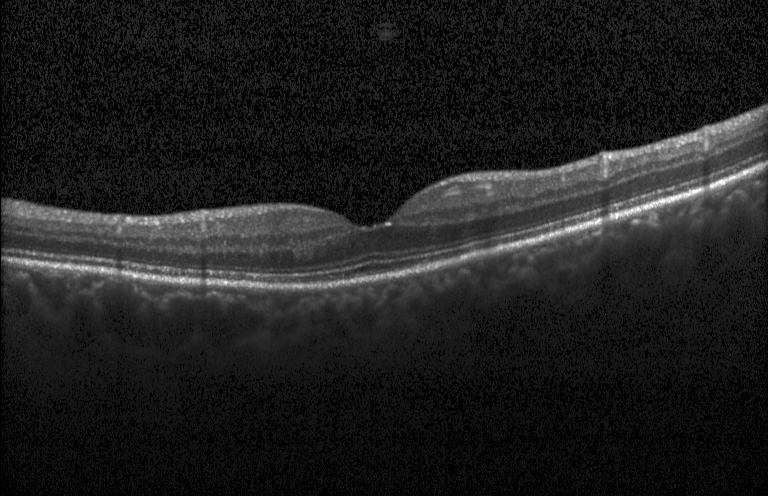
Impression: neither CNV, DME, nor drusen.